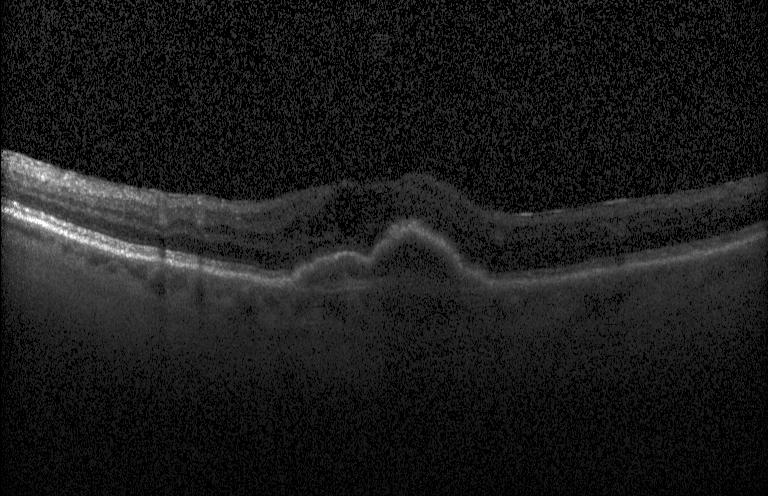
Retinal OCT B-scan; Heidelberg Spectralis OCT system. Finding: a choroidal neovascular membrane.